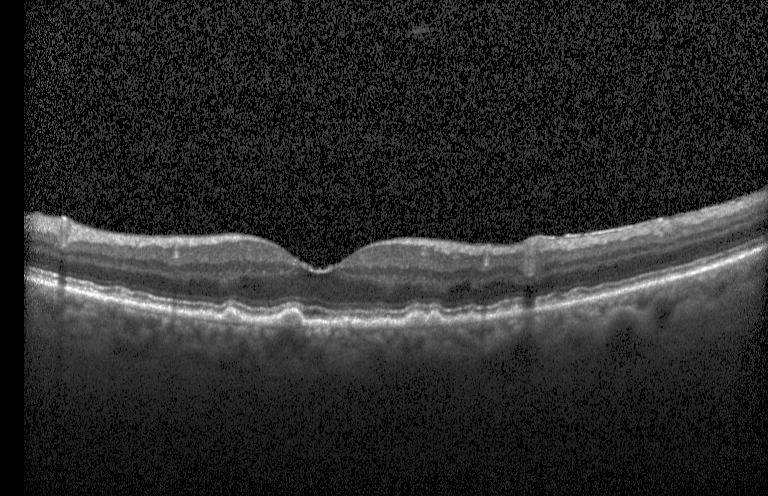 Retinal OCT cross-section showing multiple drusen.